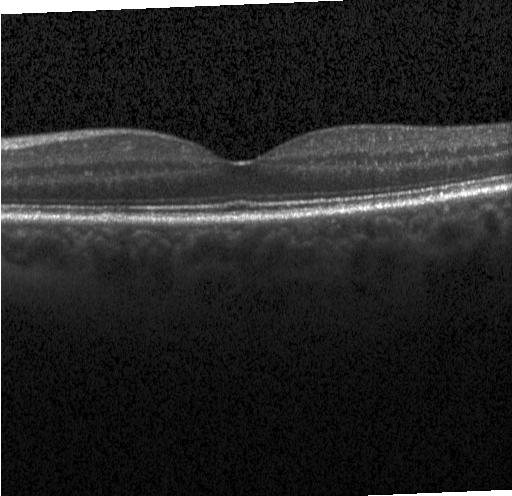
Finding: no choroidal neovascularization, diabetic macular edema, or drusen.